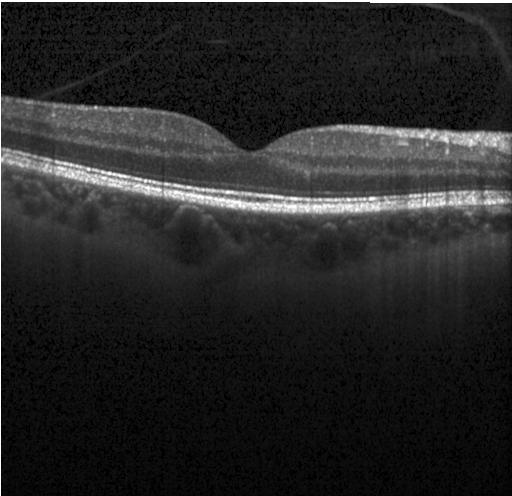 Retinal OCT cross-section
Finding: neither choroidal neovascularization, diabetic macular edema, nor drusen.